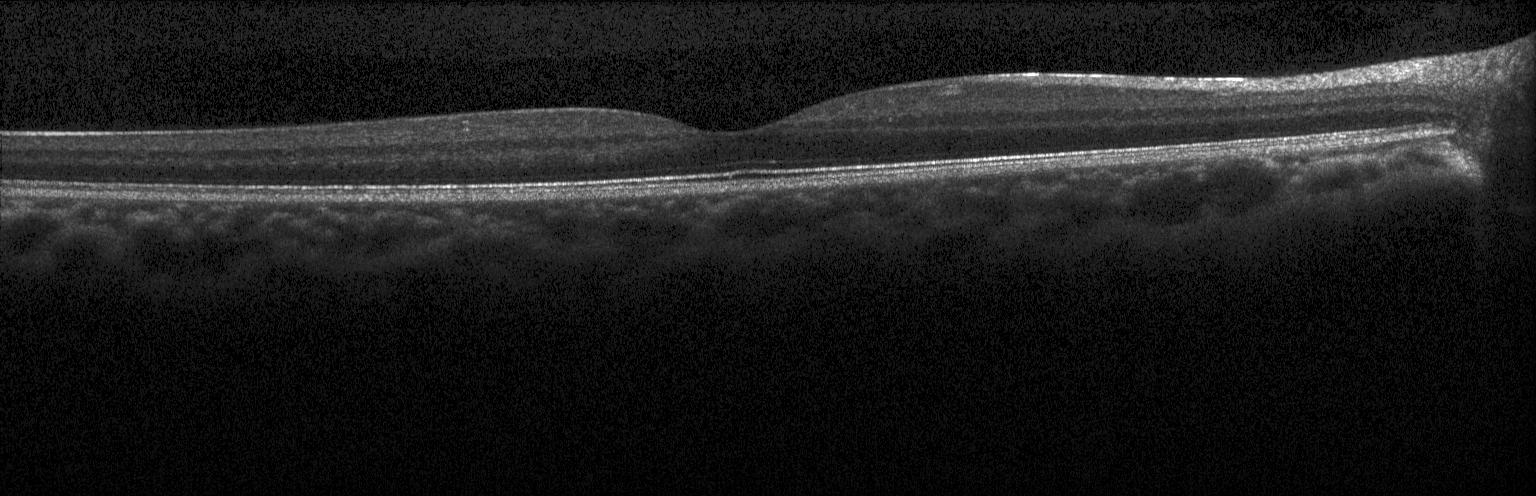
Spectral-domain OCT. Optical coherence tomography scan. Finding: neither choroidal neovascularization, diabetic macular edema, nor drusen.